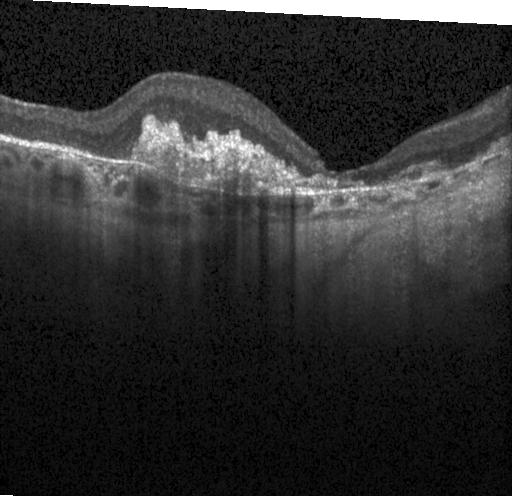 Optical coherence tomography scan, fovea-centered, spectral-domain OCT.
Diagnosis: a choroidal neovascular membrane.